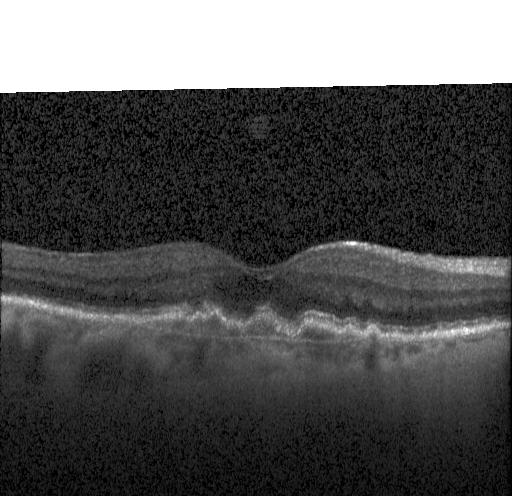 Diagnosis: choroidal neovascularization (CNV).